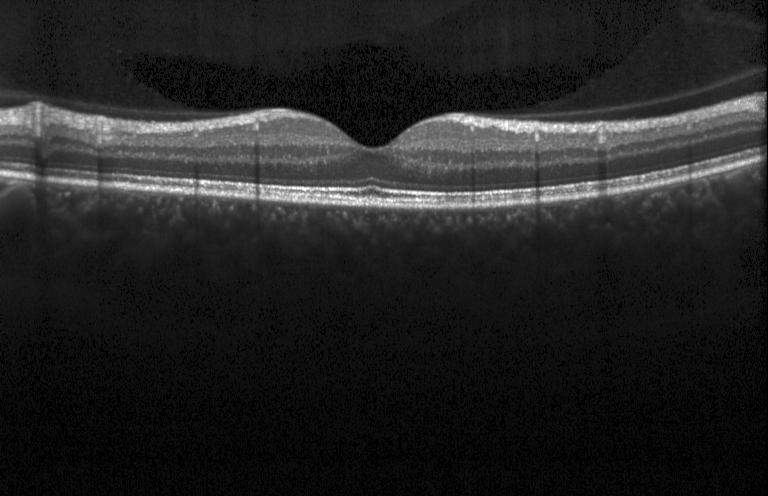
This B-scan demonstrates neither choroidal neovascularization, diabetic macular edema, nor drusen.